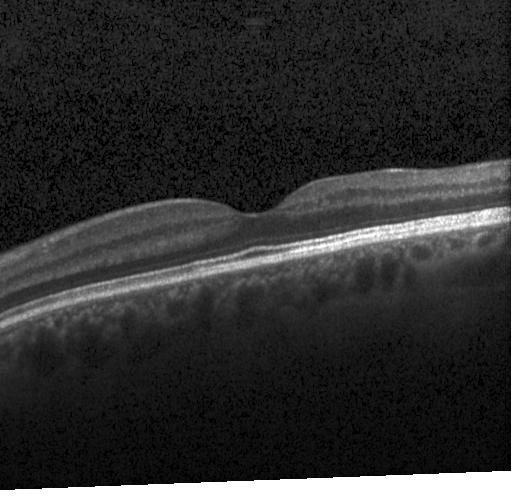 Heidelberg Spectralis OCT system · SD-OCT · OCT B-scan
Dx: no evidence of choroidal neovascularization, diabetic macular edema, or drusen.